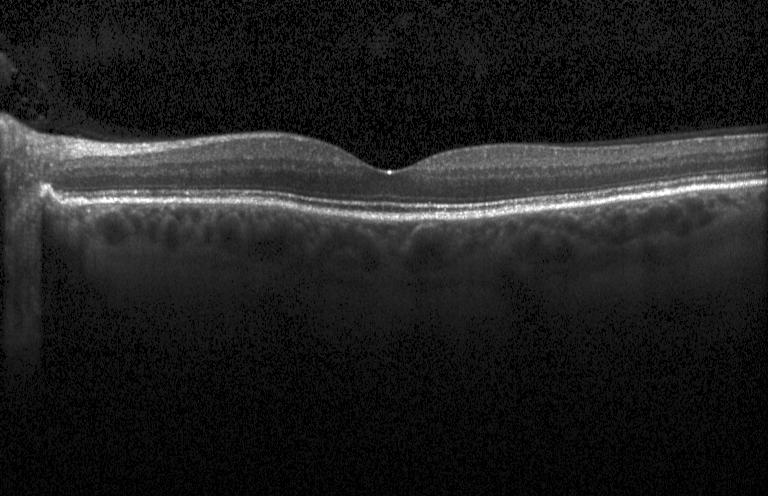 SD-OCT; horizontal scan through the fovea; OCT B-scan; Heidelberg Spectralis OCT system
Finding: neither choroidal neovascularization, diabetic macular edema, nor drusen.